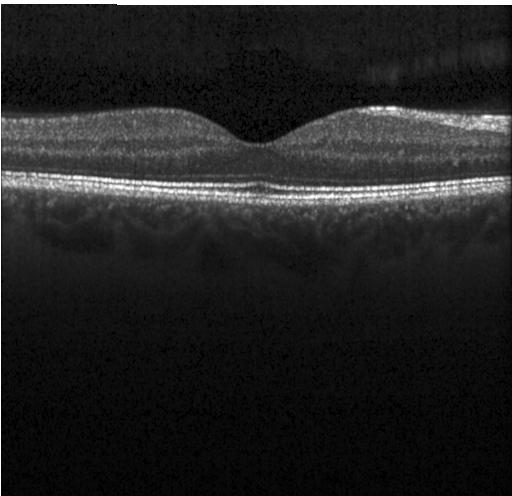

Optical coherence tomography B-scan, spectral-domain OCT, horizontal scan through the fovea.
Finding: neither choroidal neovascularization, diabetic macular edema, nor drusen.